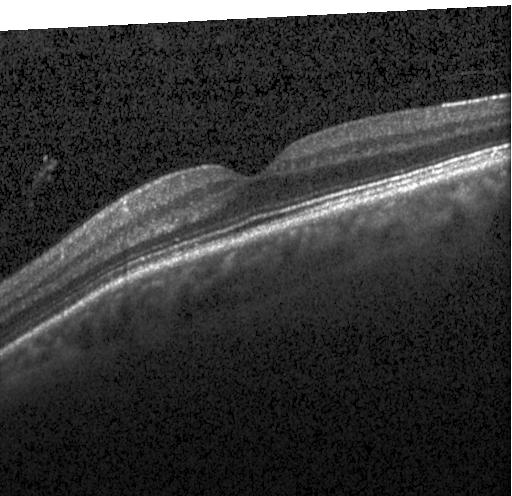

Finding: neither choroidal neovascularization, diabetic macular edema, nor drusen.